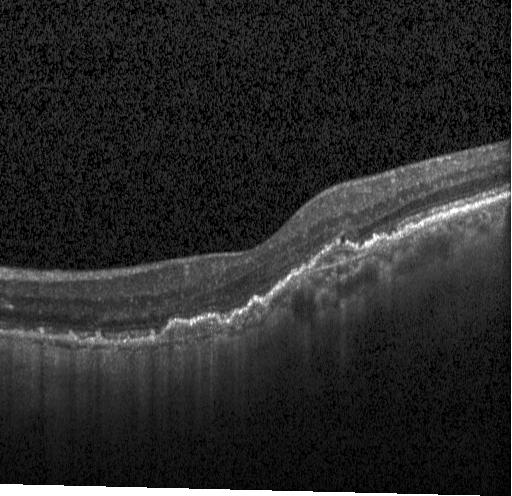
Dx: choroidal neovascularization.